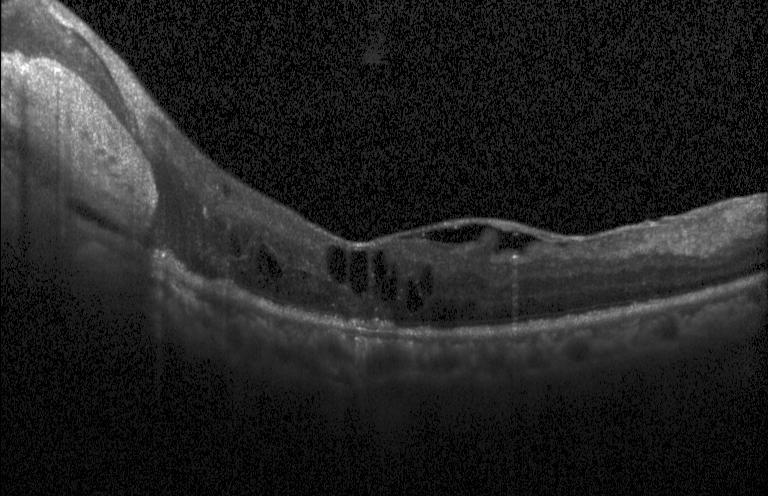 OCT line scan — The scan shows a choroidal neovascular membrane.